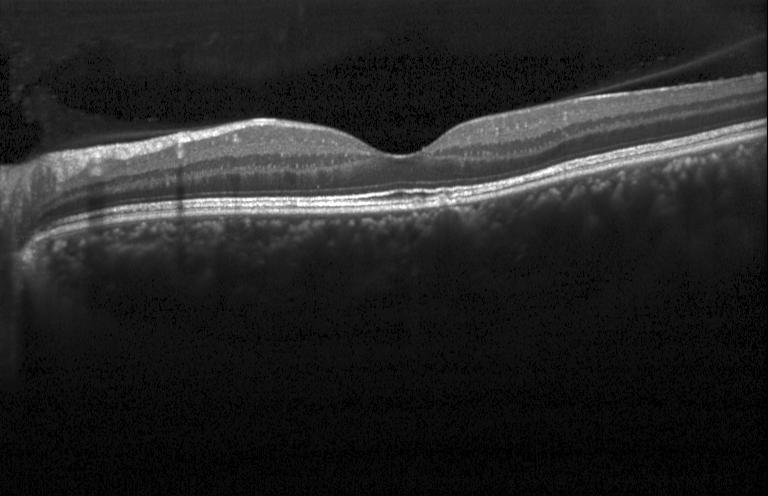

OCT B-scan · SD-OCT · Heidelberg Spectralis. Impression: no choroidal neovascularization, no diabetic macular edema, and no drusen.